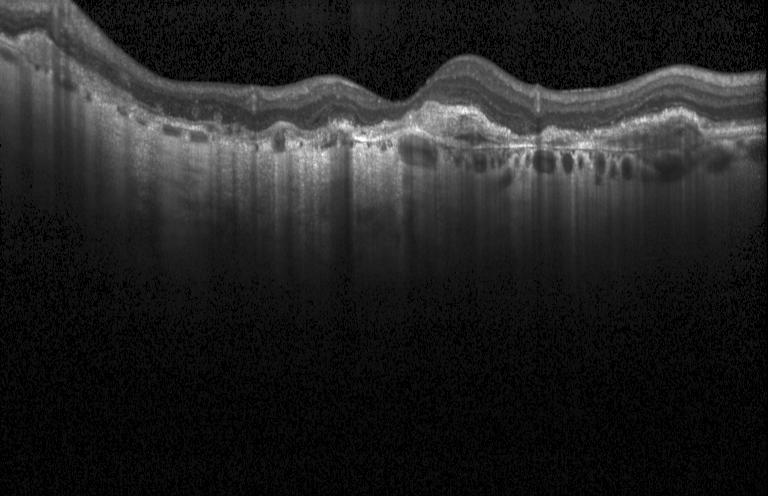 Spectral-domain optical coherence tomography, Heidelberg Spectralis, fovea-centered, optical coherence tomography scan. Dx: a choroidal neovascular membrane.